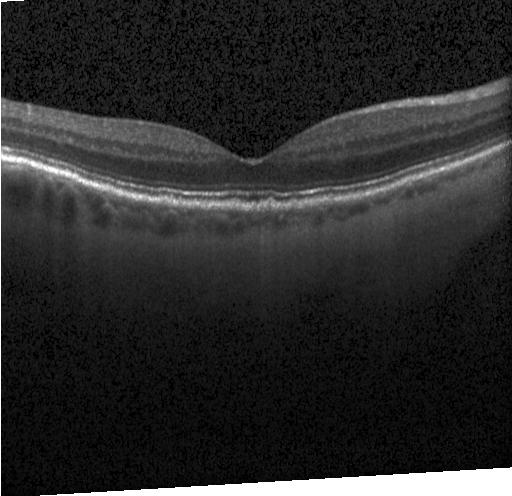 Optical coherence tomography B-scan · horizontal scan through the fovea — The scan shows drusen.